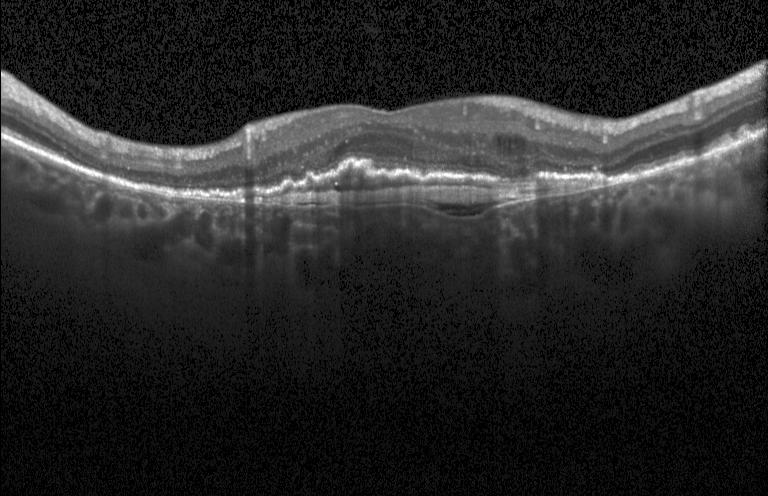
Heidelberg Spectralis; fovea-centered; spectral-domain optical coherence tomography; optical coherence tomography B-scan.
Impression: CNV.